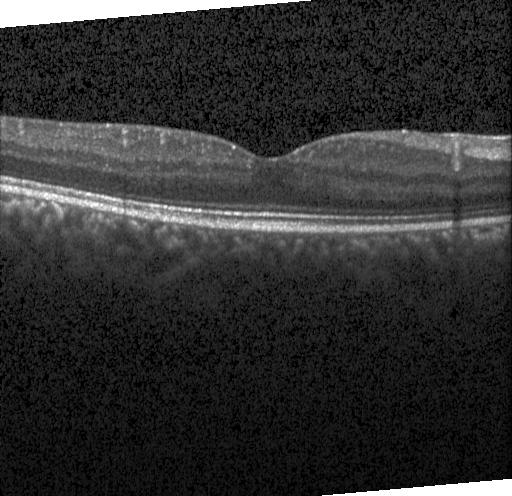
Retinal OCT cross-section · SD-OCT.
This B-scan demonstrates no choroidal neovascularization, diabetic macular edema, or drusen.